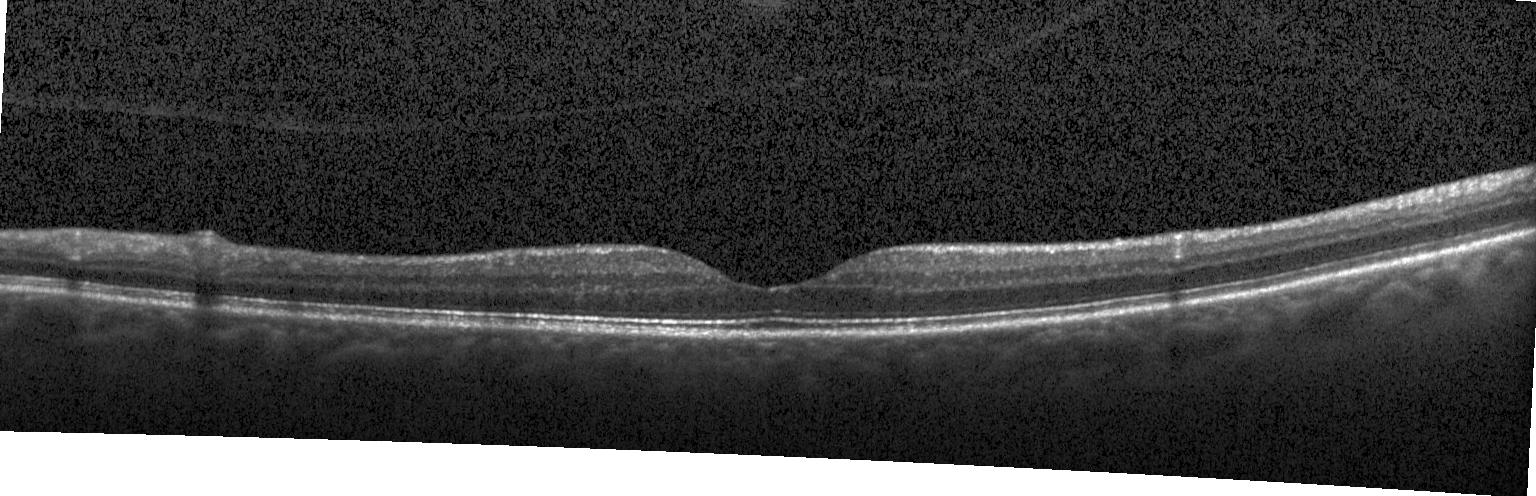
Retinal OCT B-scan, fovea-centered. No CNV, no DME, and no drusen.